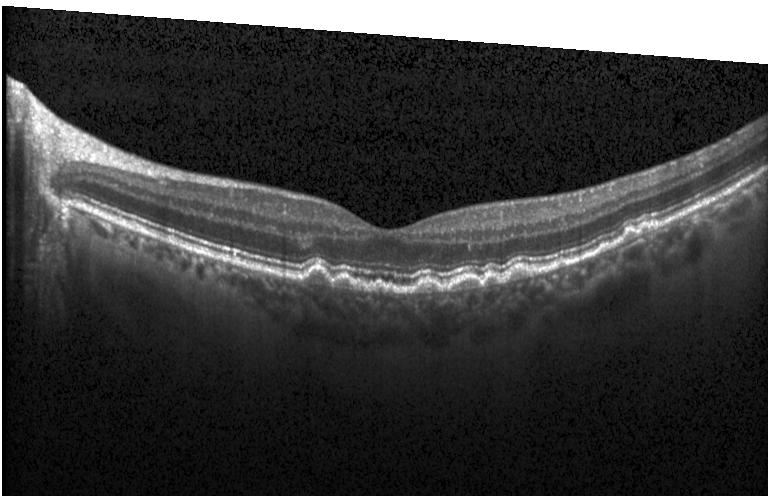

Heidelberg Spectralis; retinal OCT cross-section — Impression: drusen.